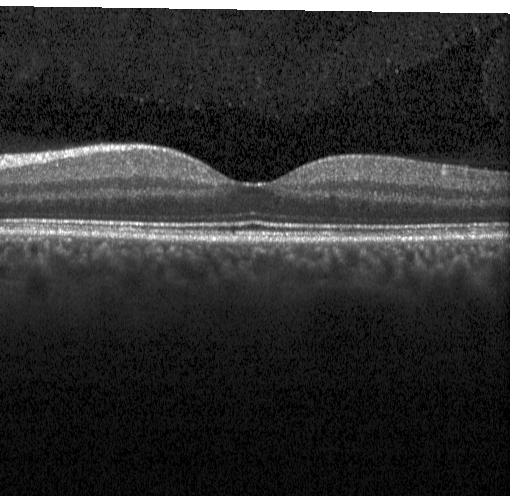 Optical coherence tomography scan. Acquired on a Heidelberg Spectralis. Centered on the fovea
Diagnosis: no choroidal neovascularization, no diabetic macular edema, and no drusen.